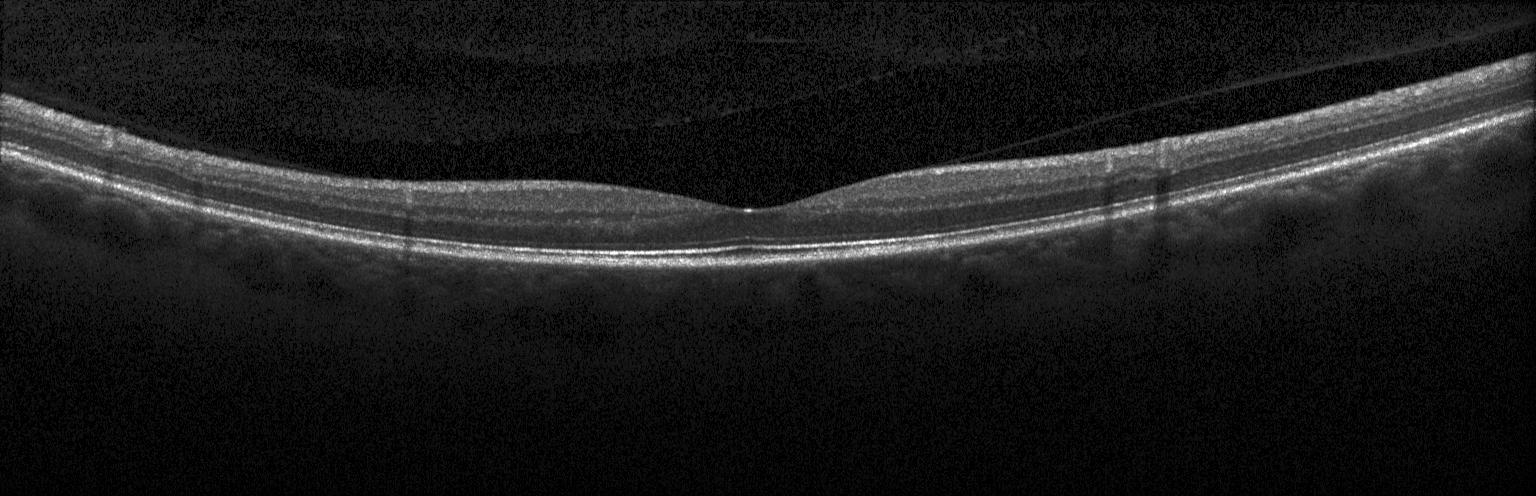
OCT finding: no CNV, no DME, and no drusen.